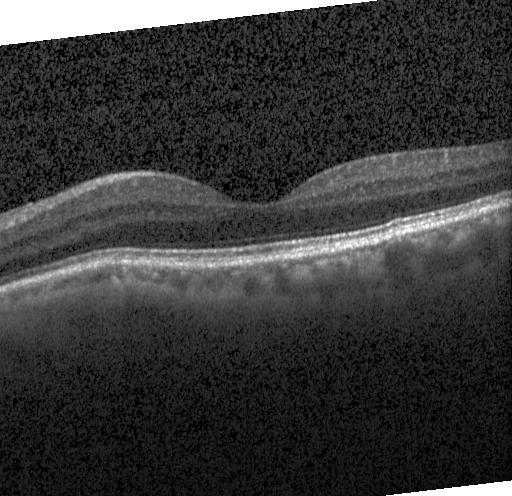 Through the macula; OCT line scan. Diagnosis: no evidence of CNV, DME, or drusen.